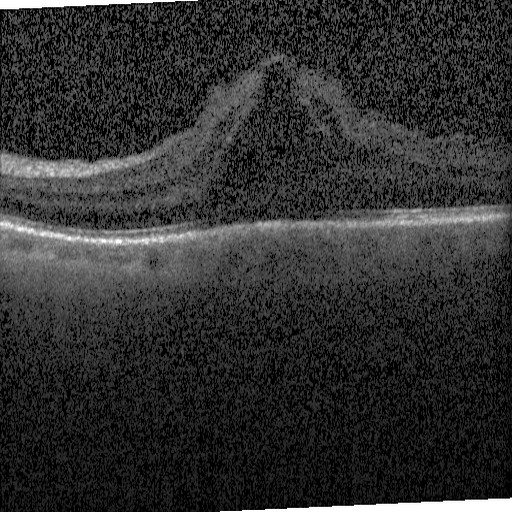
Instrument: Heidelberg Spectralis. Retinal OCT B-scan.
OCT finding: diabetic macular edema (DME).